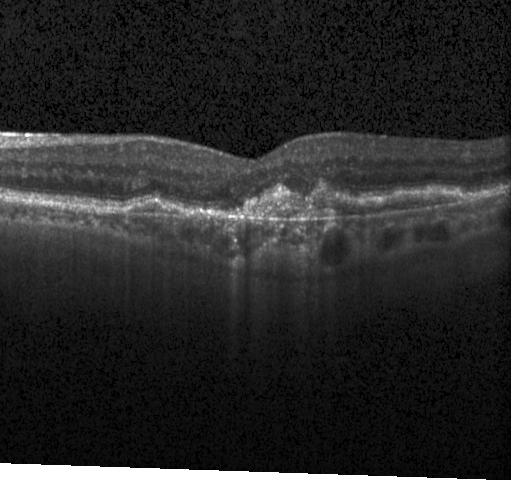
Diagnosis: a choroidal neovascular membrane.